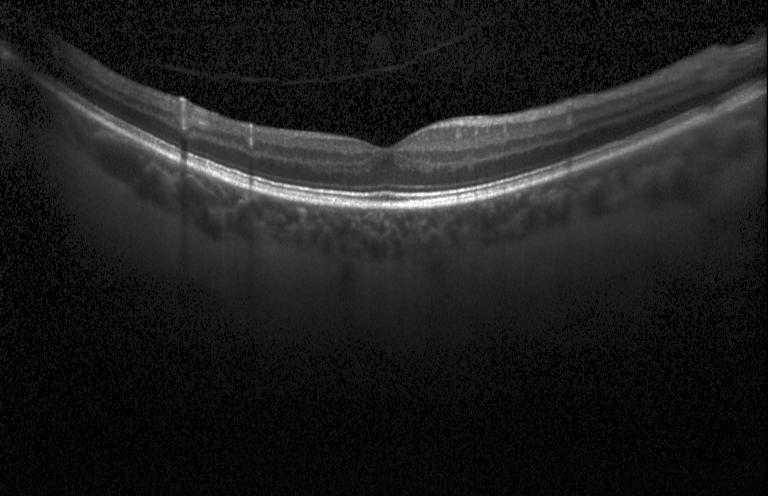
Macular scan. SD-OCT. Retinal OCT cross-section
Assessment: no CNV, no DME, and no drusen.